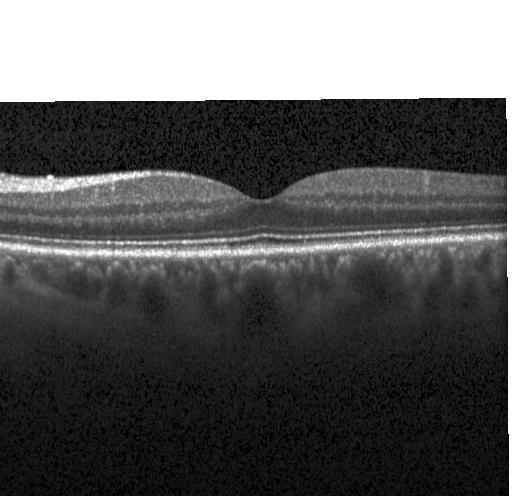
Optical coherence tomography B-scan
Impression: no CNV, no DME, and no drusen.